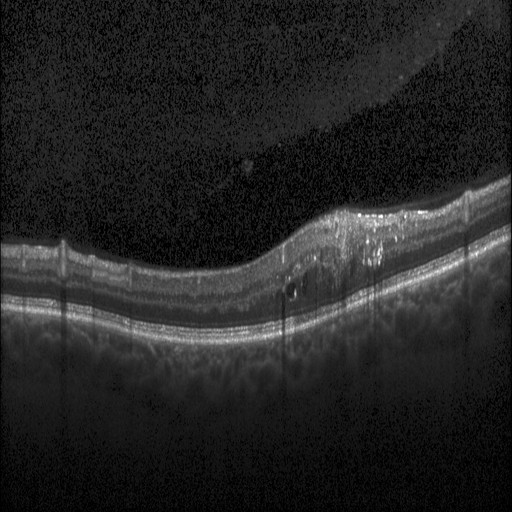
OCT line scan; spectral-domain optical coherence tomography; Heidelberg Spectralis.
Finding: DME.